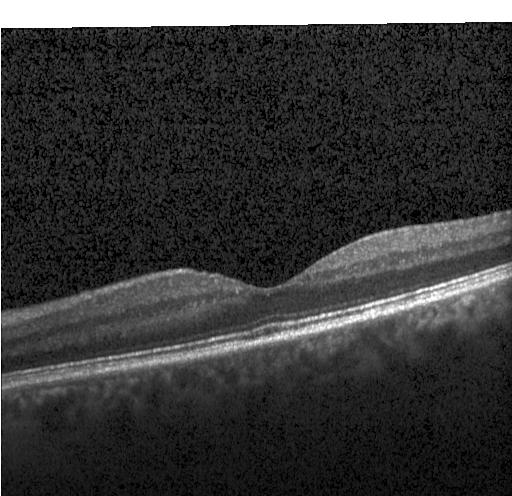
Retinal OCT cross-section, instrument: Heidelberg Spectralis. The scan shows neither choroidal neovascularization, diabetic macular edema, nor drusen.